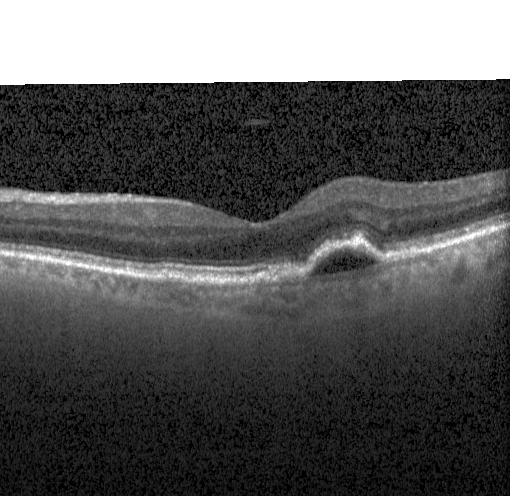

Dx: a choroidal neovascular membrane.